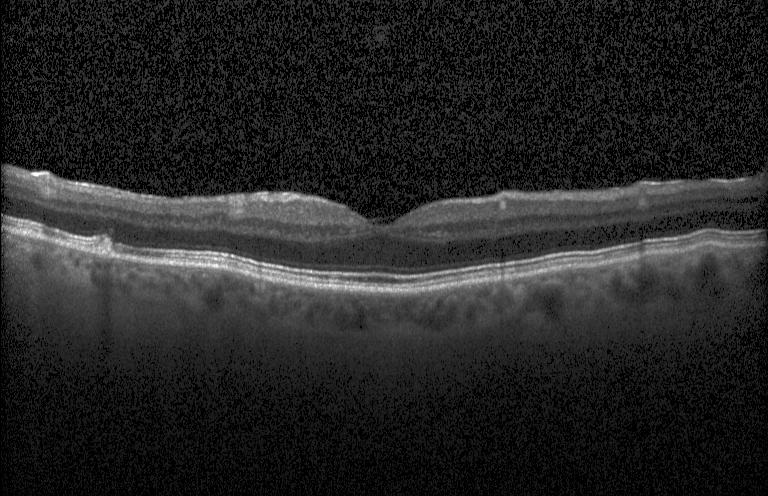
SD-OCT · macular scan · OCT B-scan
OCT finding: sub-RPE drusenoid deposits.